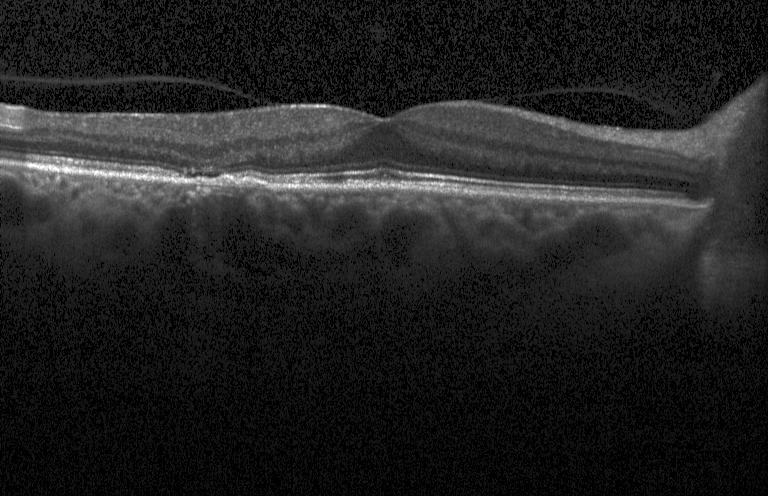
Spectral-domain OCT B-scan: choroidal neovascularization.